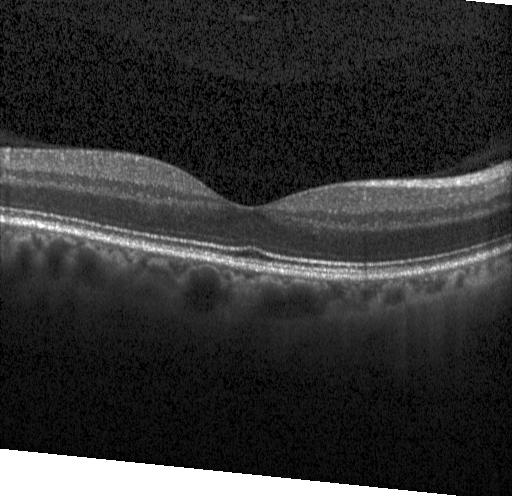
Macular scan. OCT line scan. Spectral-domain optical coherence tomography. Macular OCT: no evidence of choroidal neovascularization, diabetic macular edema, or drusen.